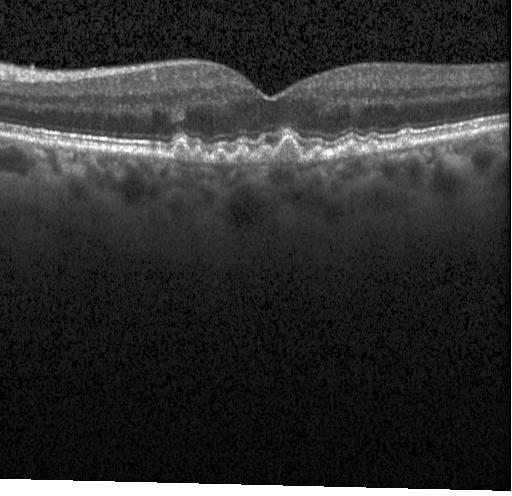

Finding: multiple drusen.